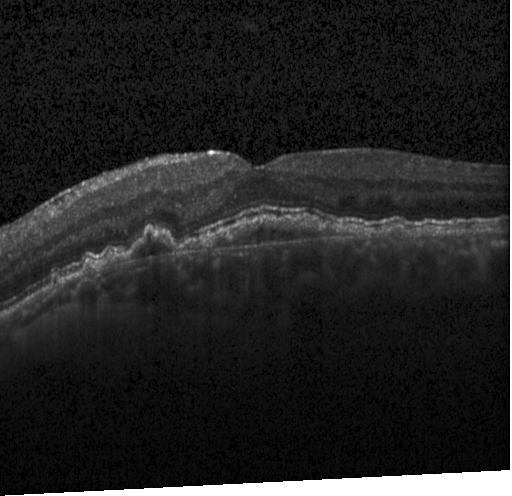

Acquired on a Heidelberg Spectralis, optical coherence tomography scan
Assessment: a choroidal neovascular membrane.